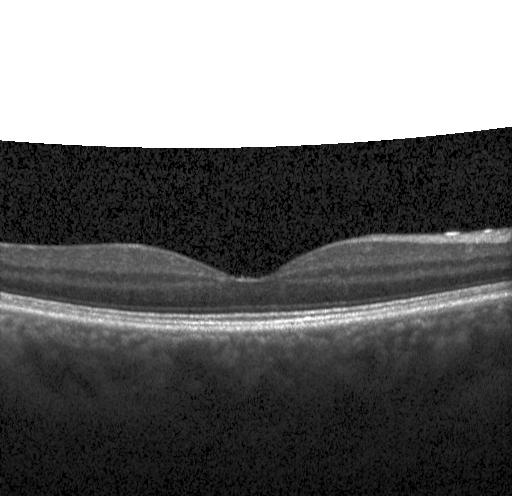 SD-OCT. Fovea-centered. Retinal OCT cross-section — Assessment: no evidence of CNV, DME, or drusen.